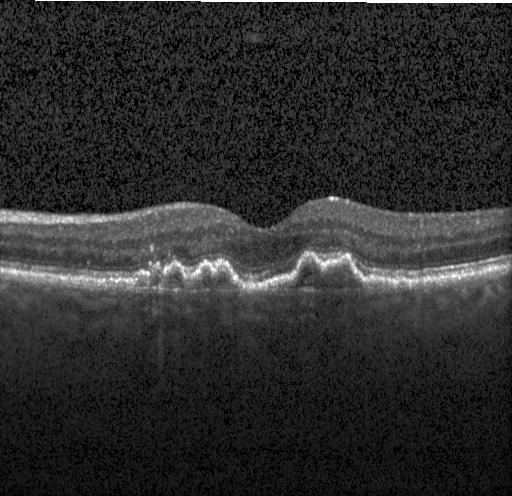

Spectral-domain OCT · Heidelberg Spectralis · optical coherence tomography B-scan. Finding: a choroidal neovascular membrane.